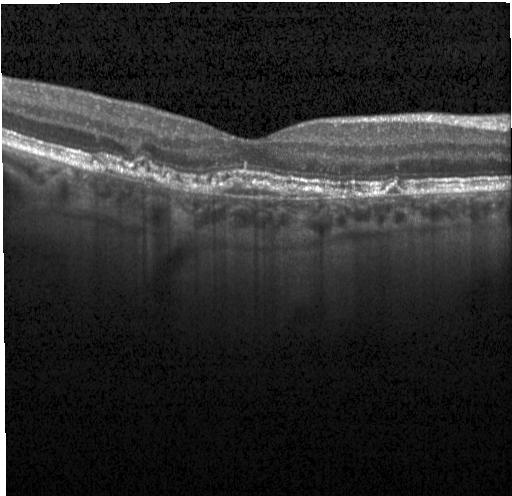 Impression: a choroidal neovascular membrane.